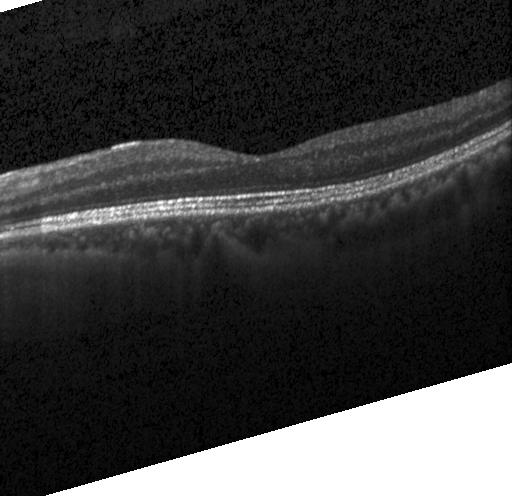 OCT line scan. This B-scan demonstrates no choroidal neovascularization, no diabetic macular edema, and no drusen.